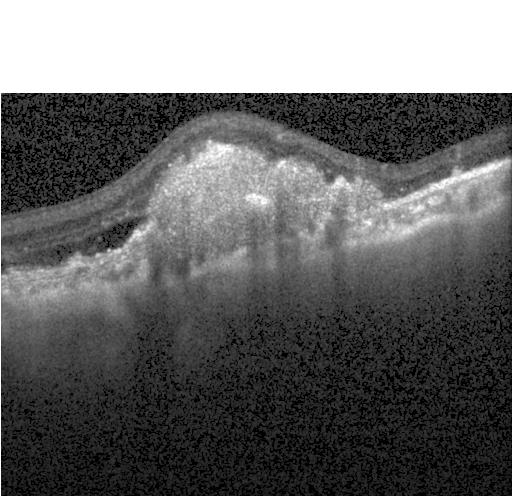
OCT line scan — Diagnosis: CNV.